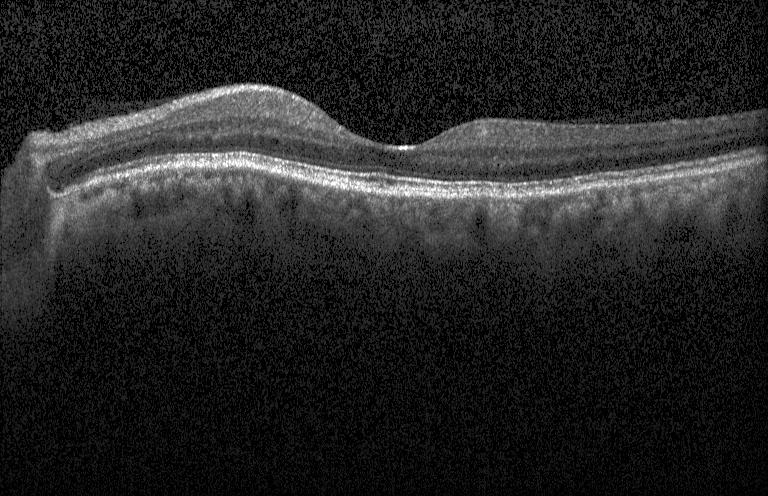

Macular OCT demonstrating no choroidal neovascularization, diabetic macular edema, or drusen.